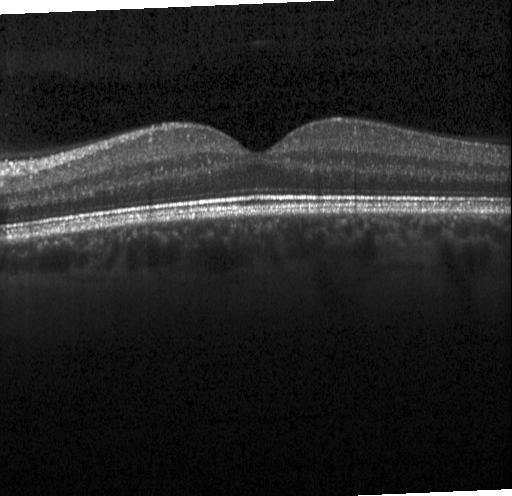

Optical coherence tomography scan — Macular OCT: neither choroidal neovascularization, diabetic macular edema, nor drusen.